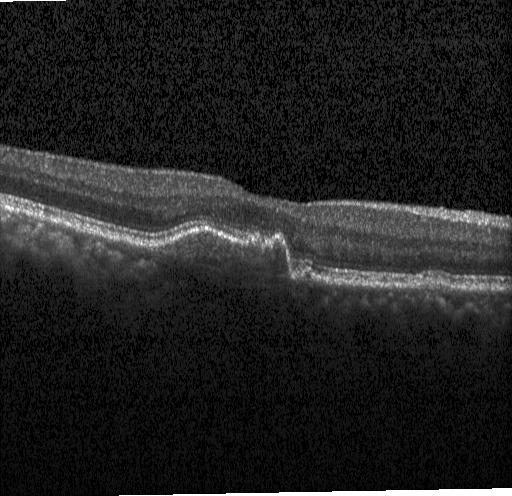 Fovea-centered. Optical coherence tomography scan
Finding: drusen.